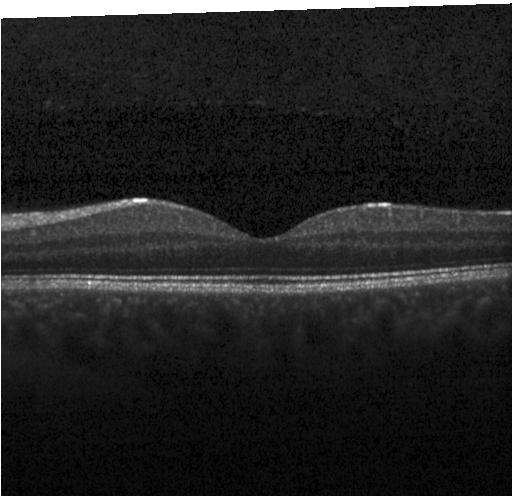
Diagnosis: neither choroidal neovascularization, diabetic macular edema, nor drusen.